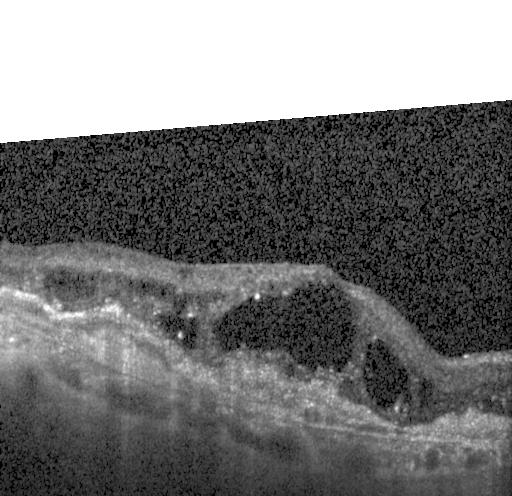

OCT line scan. Spectral-domain optical coherence tomography. Heidelberg Spectralis OCT system. Horizontal scan through the fovea.
Macular OCT: a choroidal neovascular membrane.